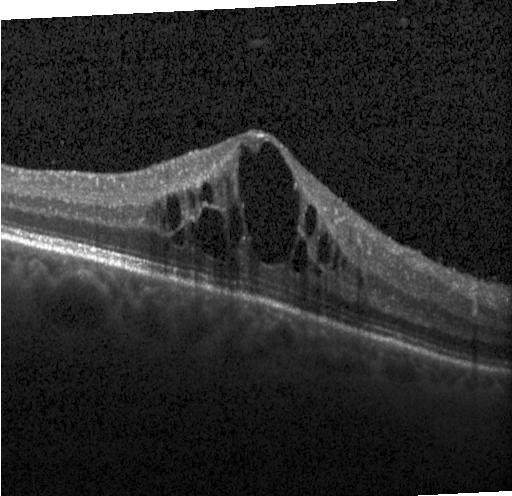
OCT B-scan showing DME.